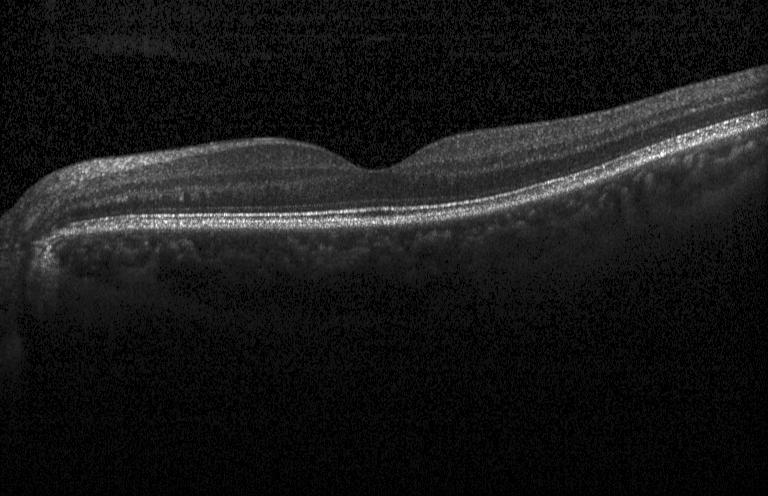

Macular OCT demonstrating no choroidal neovascularization, diabetic macular edema, or drusen.